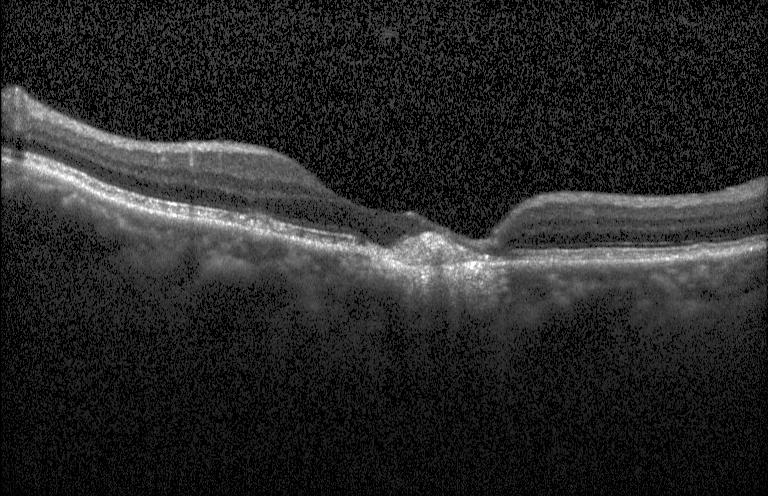

Assessment: choroidal neovascularization (CNV).